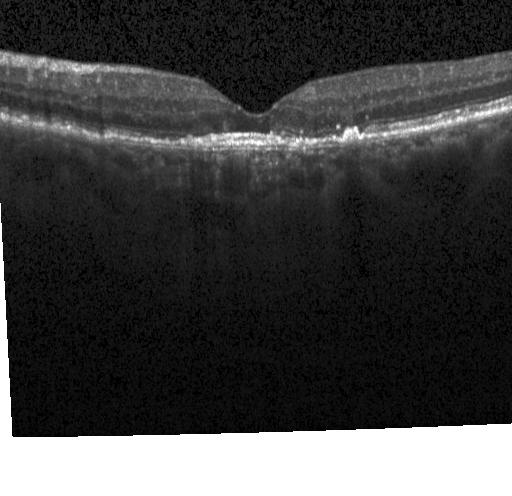 Retinal OCT B-scan.
Diagnosis: CNV.